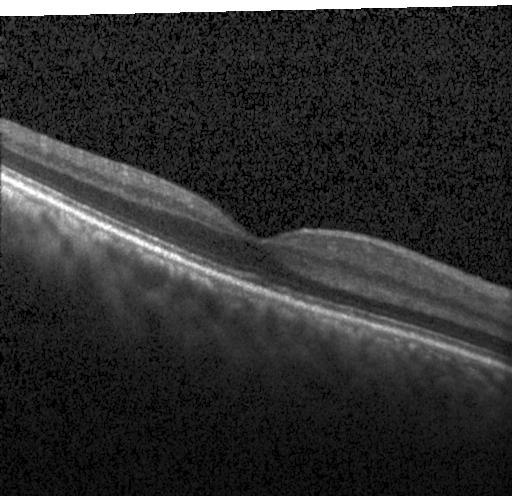

Assessment: no CNV, DME, or drusen.